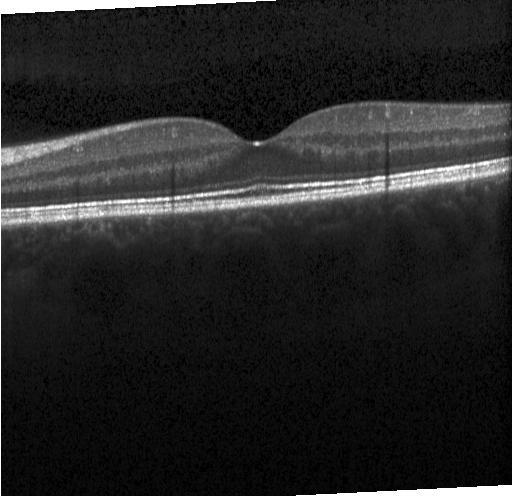
OCT scan showing no CNV, DME, or drusen.